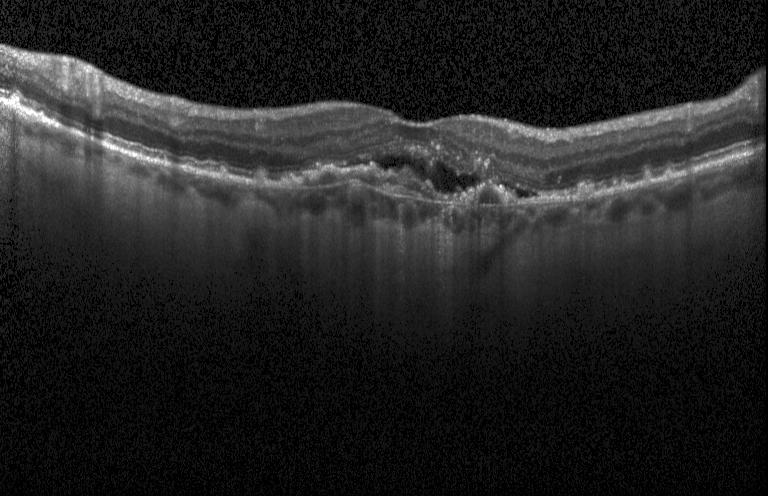 Diagnosis: choroidal neovascularization.